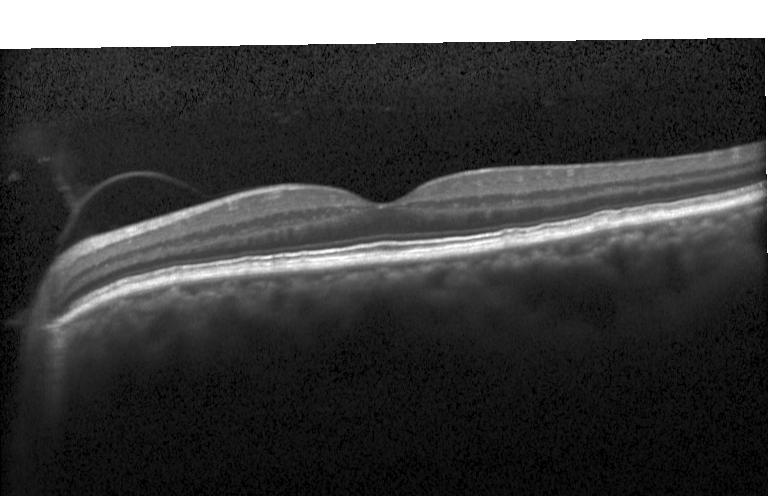

Optical coherence tomography B-scan. Macular scan. Acquired on a Heidelberg Spectralis. Impression: neither CNV, DME, nor drusen.